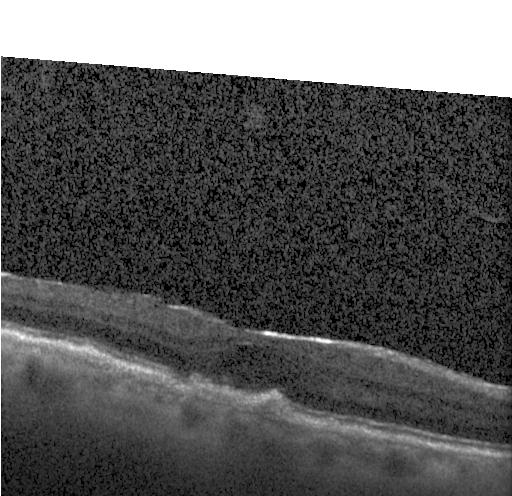

Optical coherence tomography B-scan; fovea-centered; spectral-domain optical coherence tomography; acquired on a Heidelberg Spectralis. Assessment: CNV.